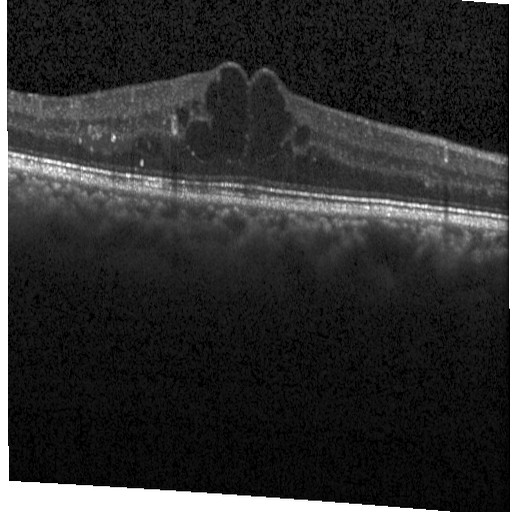 Spectral-domain OCT B-scan: diabetic macular edema.